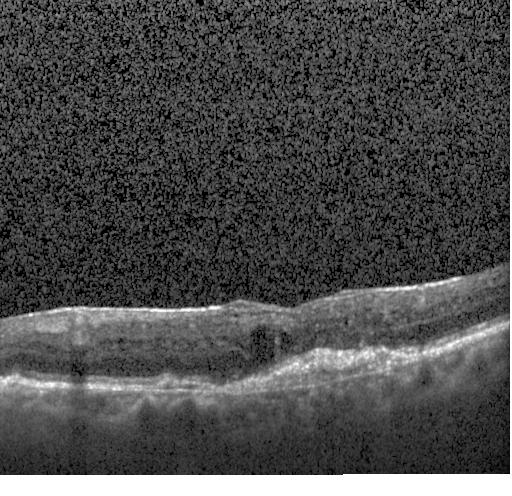
SD-OCT. Horizontal scan through the fovea. Optical coherence tomography scan. Heidelberg Spectralis. Diagnosis: a choroidal neovascular membrane.